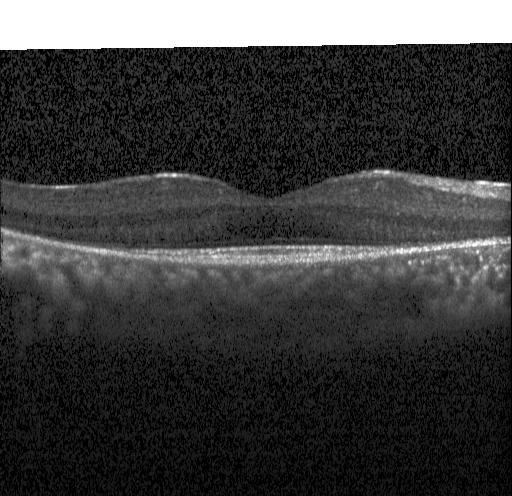 Assessment: neither CNV, DME, nor drusen.